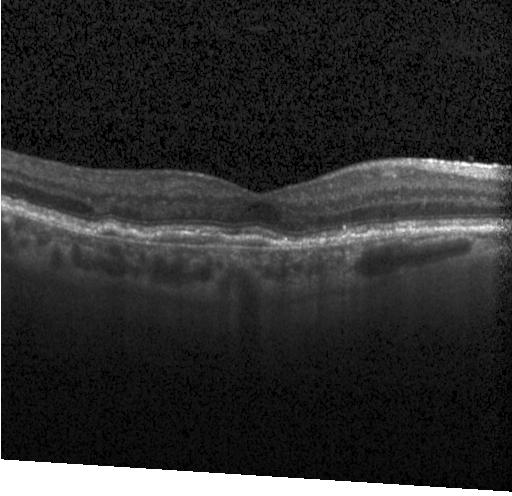
The scan shows choroidal neovascularization.